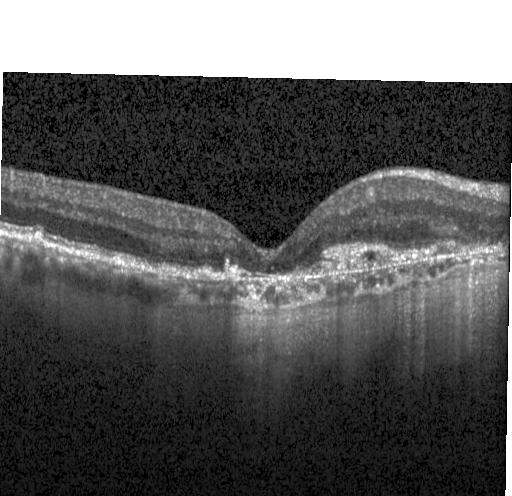
This B-scan demonstrates a choroidal neovascular membrane.